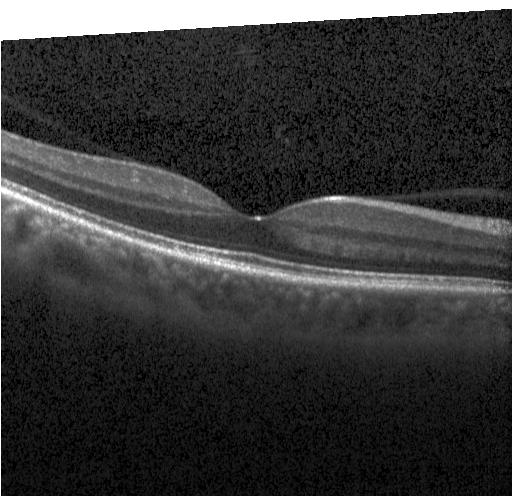

Acquired on a Heidelberg Spectralis; retinal OCT B-scan.
Impression: no evidence of CNV, DME, or drusen.